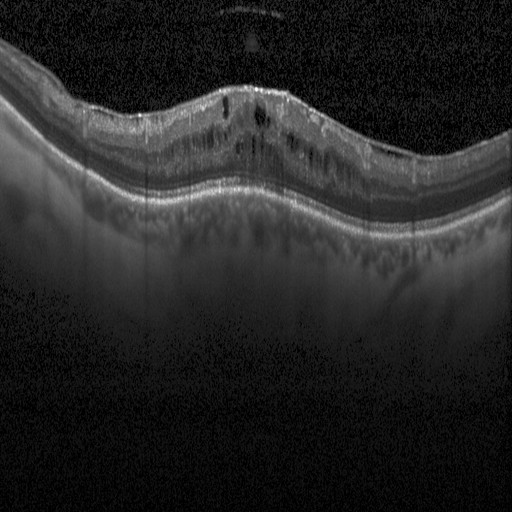

OCT B-scan; instrument: Heidelberg Spectralis; spectral-domain OCT
Impression: diabetic macular edema (DME).